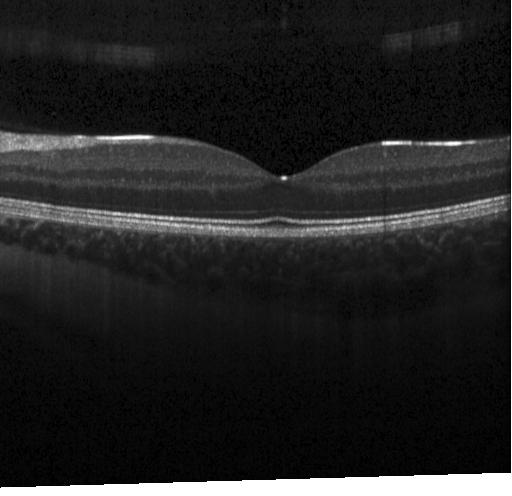
Fovea-centered · OCT line scan · spectral-domain OCT · instrument: Heidelberg Spectralis
Assessment: no choroidal neovascularization, no diabetic macular edema, and no drusen.